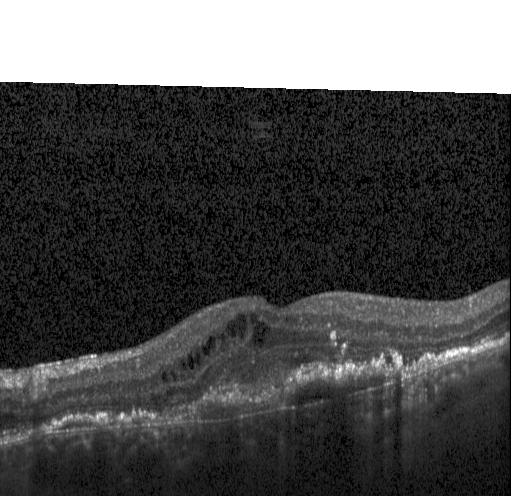
Spectral-domain optical coherence tomography, horizontal scan through the fovea, OCT line scan, instrument: Heidelberg Spectralis. This B-scan demonstrates a choroidal neovascular membrane.